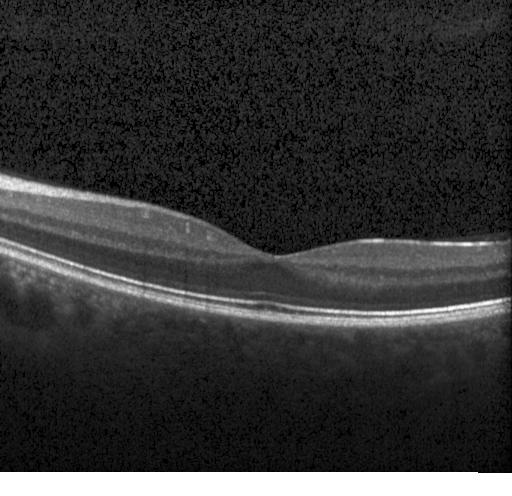

OCT B-scan showing no choroidal neovascularization, diabetic macular edema, or drusen.